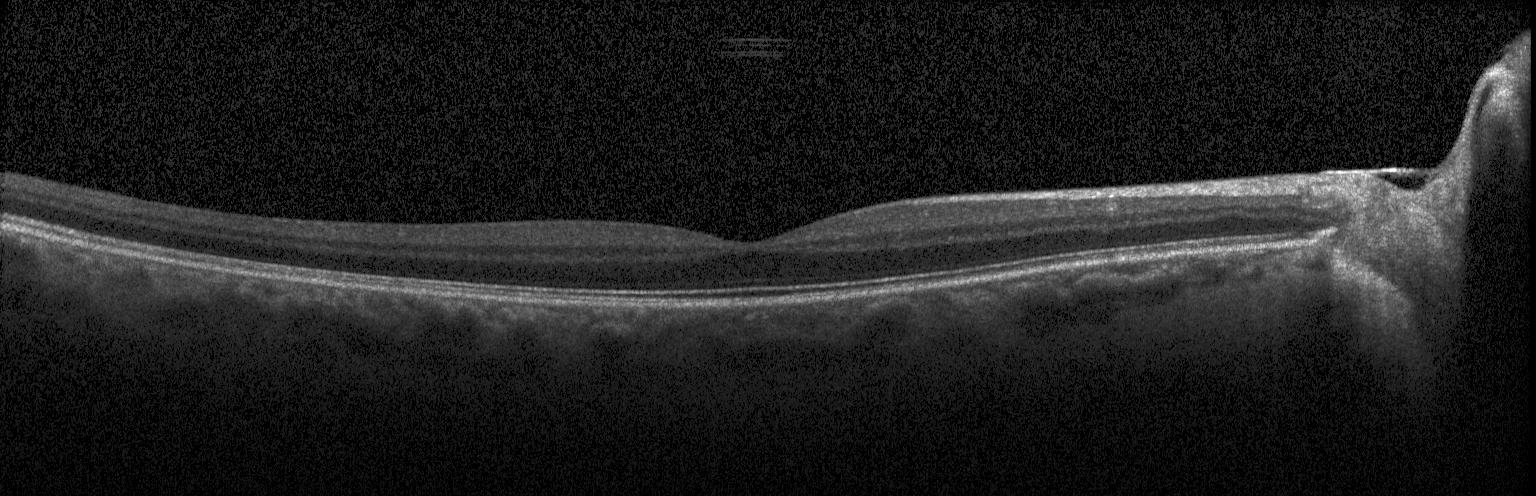

Finding: no choroidal neovascularization, no diabetic macular edema, and no drusen.